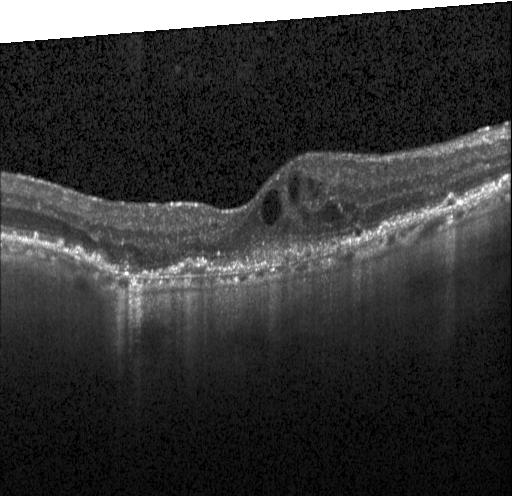

Optical coherence tomography B-scan; Heidelberg Spectralis OCT system; horizontal scan through the fovea.
OCT finding: a choroidal neovascular membrane.